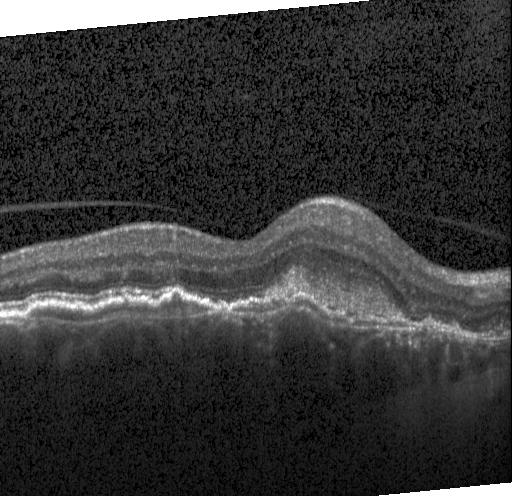

Retinal OCT cross-section. Diagnosis: choroidal neovascularization (CNV).